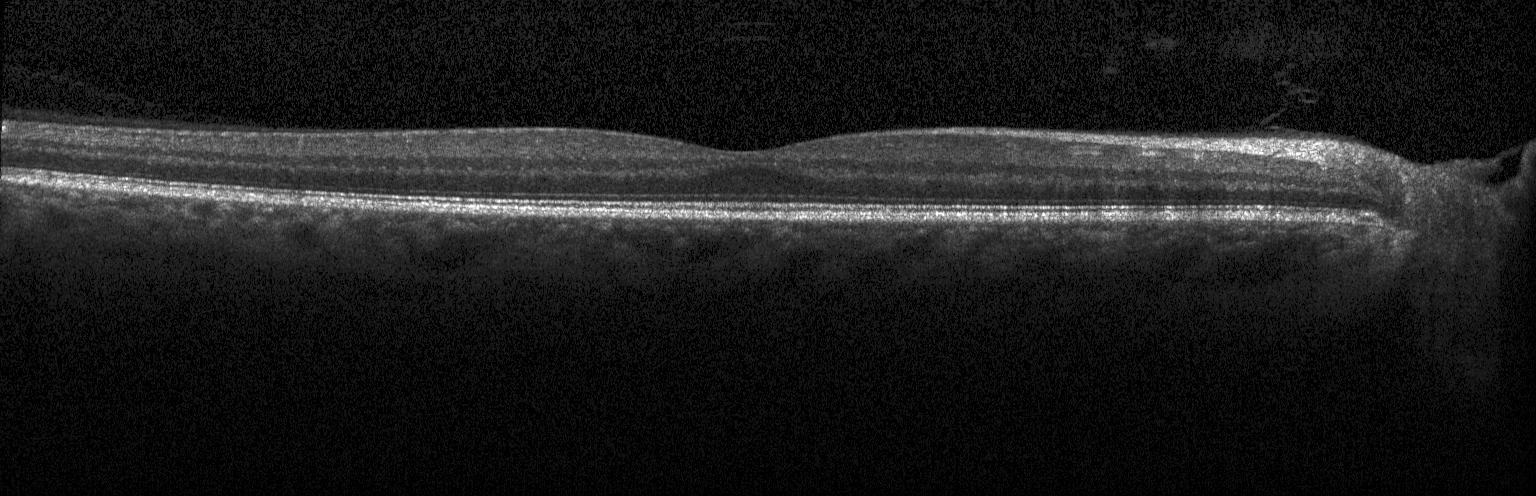 Optical coherence tomography B-scan · Heidelberg Spectralis OCT system
OCT finding: no evidence of choroidal neovascularization, diabetic macular edema, or drusen.